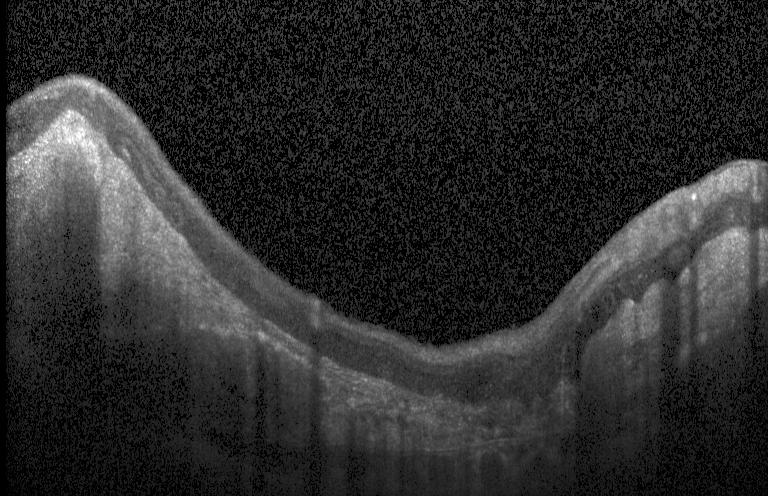

Spectral-domain OCT B-scan: CNV.